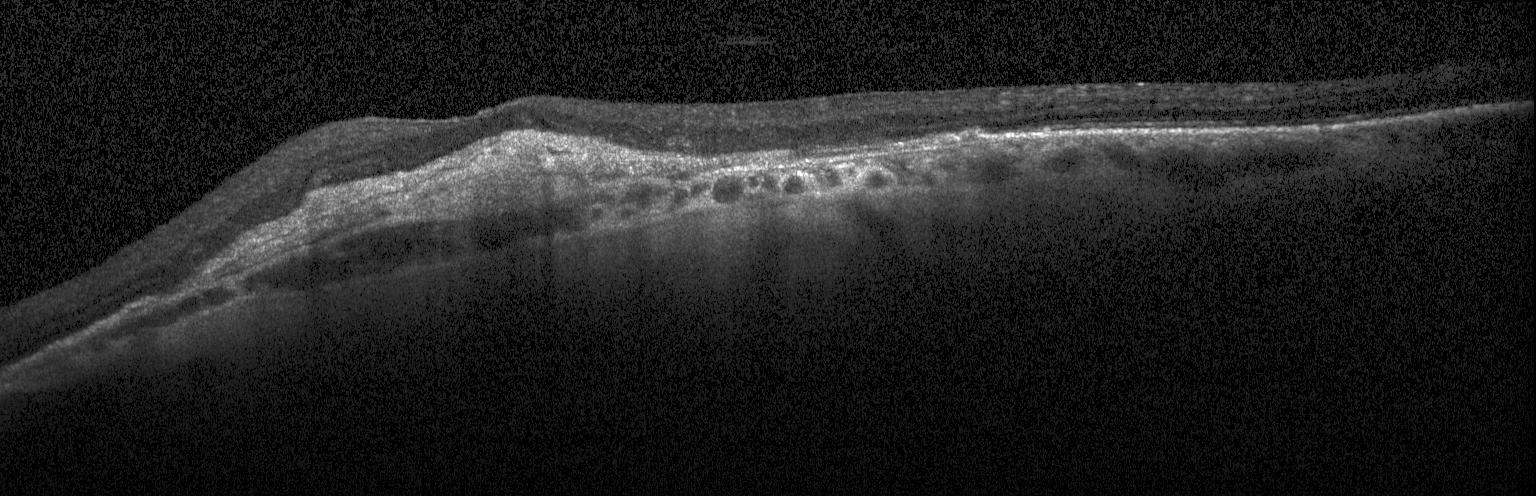 OCT B-scan · SD-OCT. This B-scan demonstrates CNV.